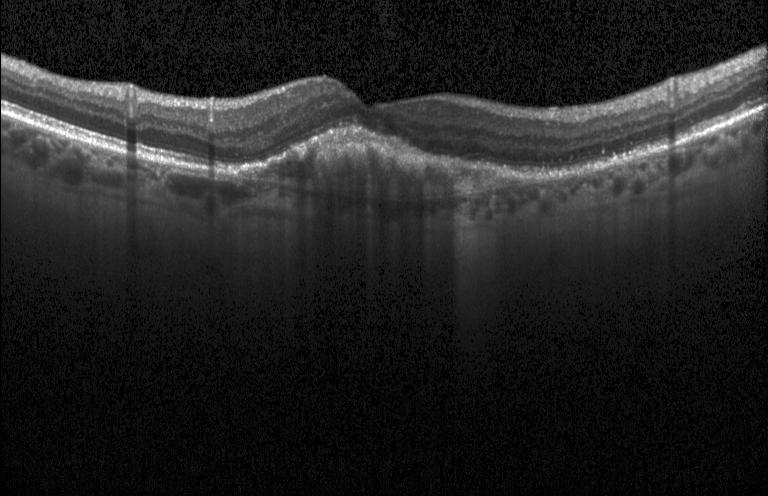 Impression: a choroidal neovascular membrane.